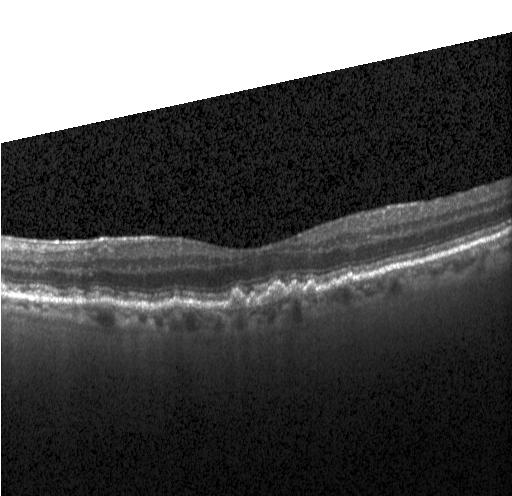 Retinal OCT cross-section showing drusen.